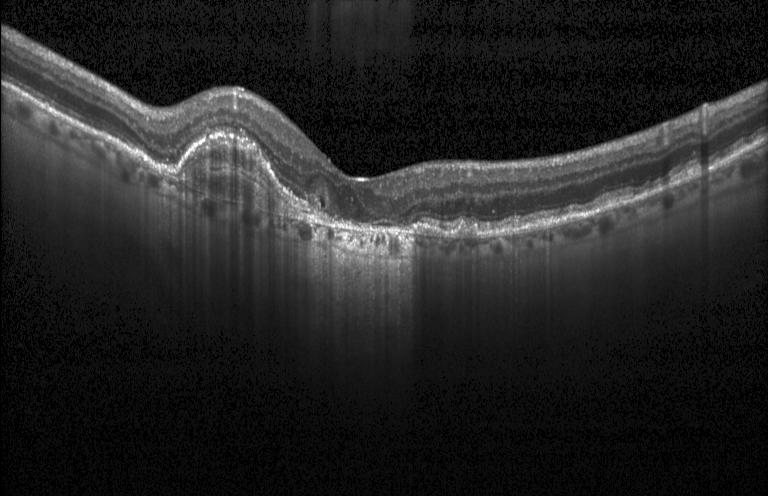
Retinal OCT cross-section.
This B-scan demonstrates choroidal neovascularization.